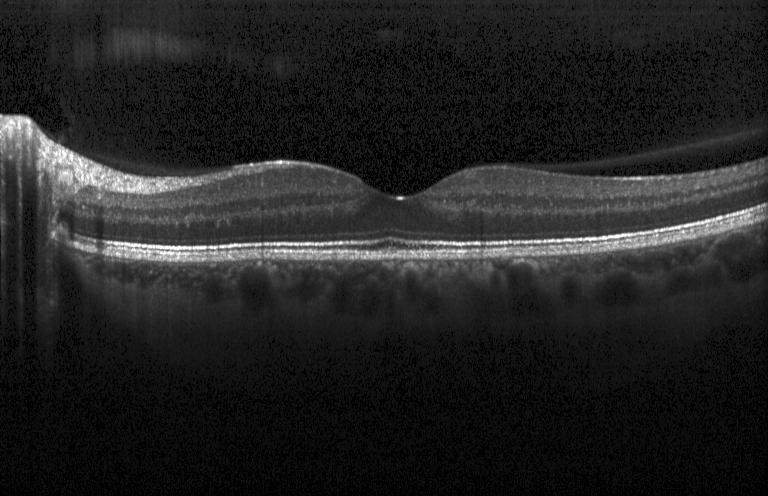
Macular OCT: no choroidal neovascularization, no diabetic macular edema, and no drusen.